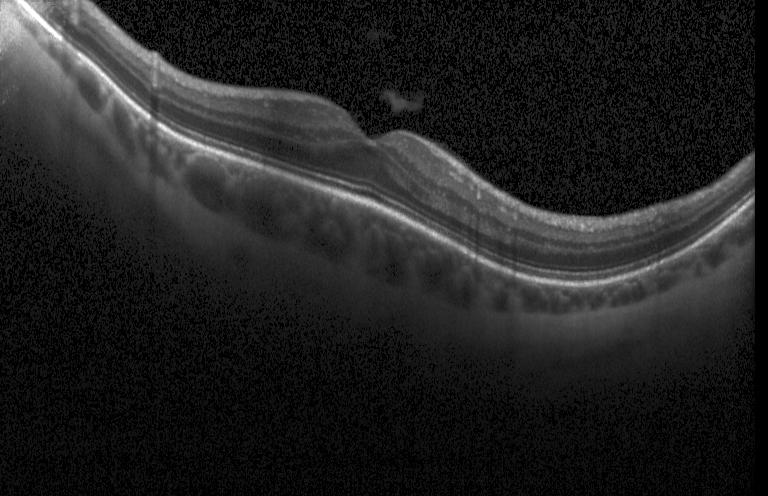 Acquired on a Heidelberg Spectralis. OCT line scan. Spectral-domain optical coherence tomography. Centered on the fovea. Dx: no evidence of choroidal neovascularization, diabetic macular edema, or drusen.